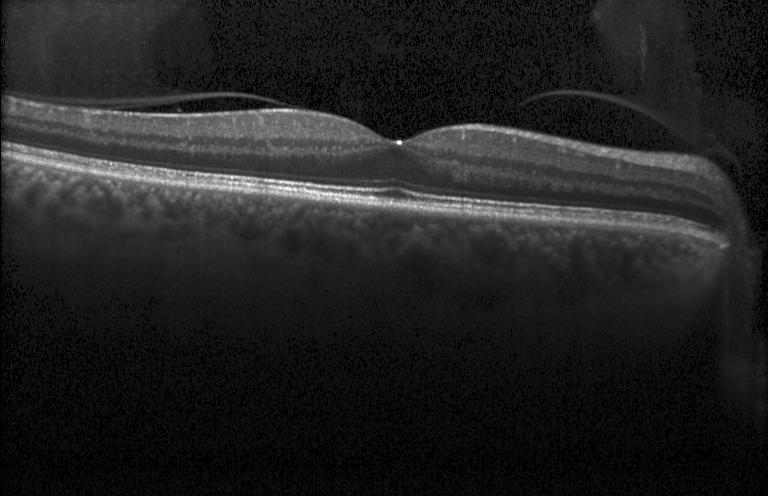

Retinal OCT cross-section; spectral-domain OCT; instrument: Heidelberg Spectralis
Assessment: no CNV, no DME, and no drusen.